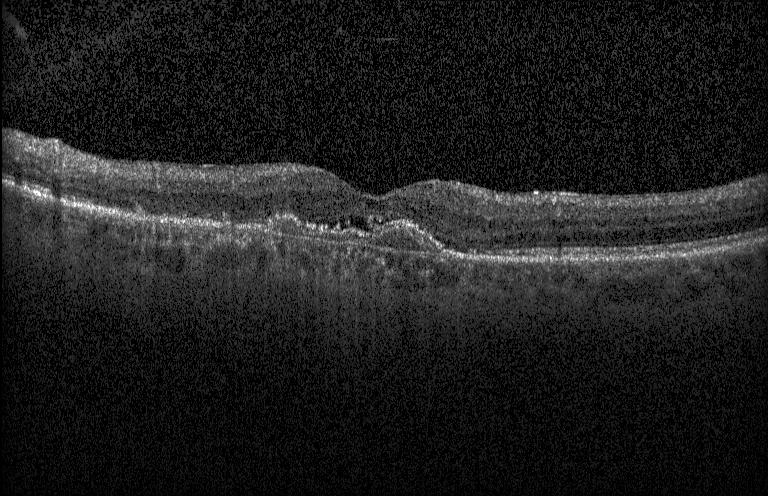

Spectral-domain OCT · retinal OCT cross-section. The scan shows a choroidal neovascular membrane.